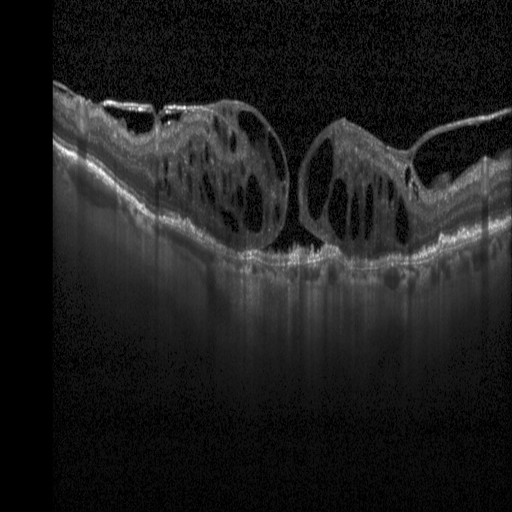
Impression: diabetic macular edema.